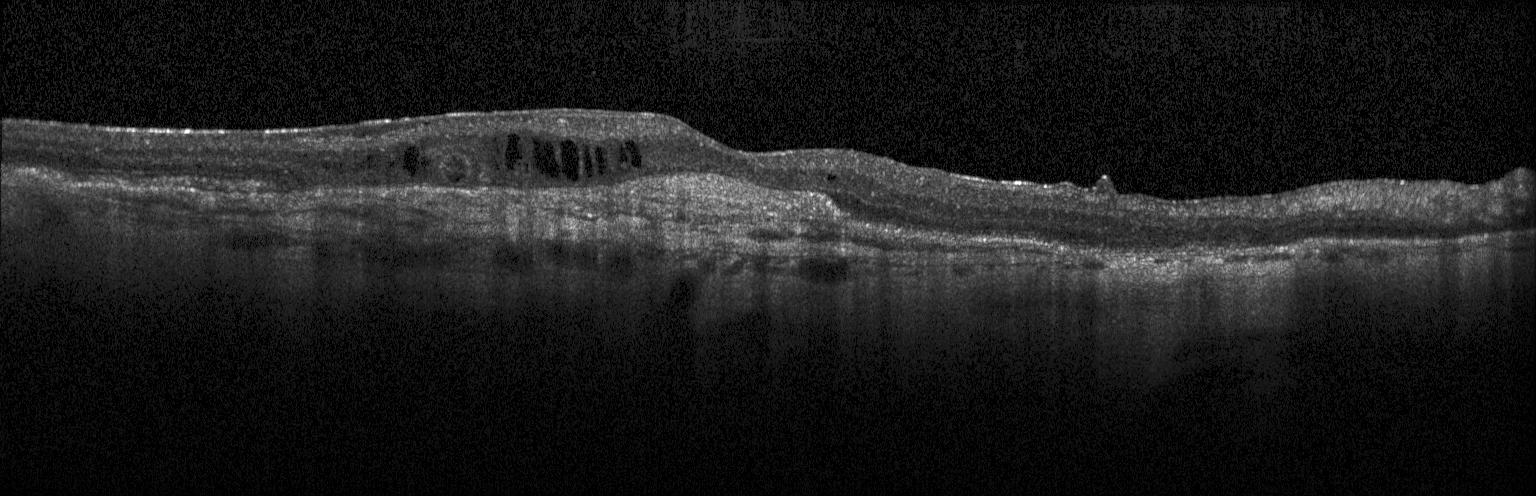

Diagnosis: a choroidal neovascular membrane.